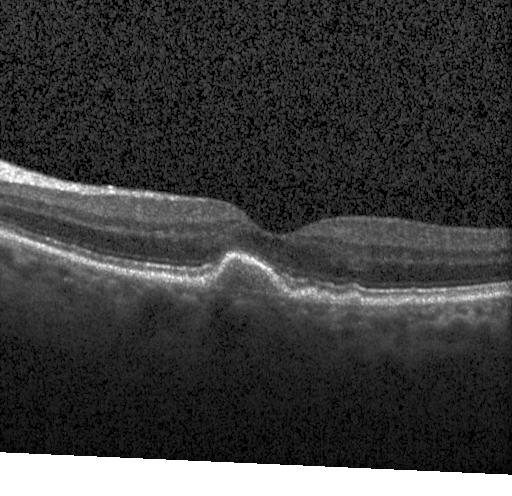

SD-OCT · horizontal scan through the fovea · optical coherence tomography B-scan — Diagnosis: multiple drusen.